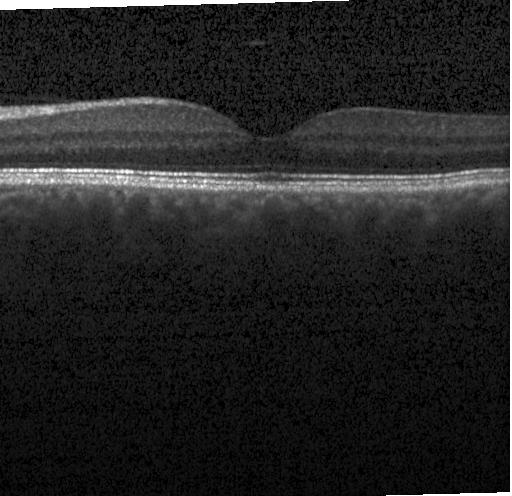

Macular OCT: no evidence of choroidal neovascularization, diabetic macular edema, or drusen.